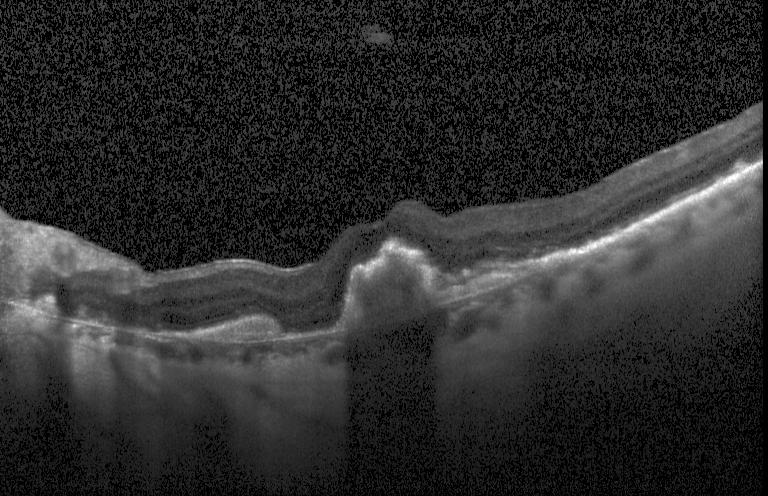 Macular OCT demonstrating CNV.